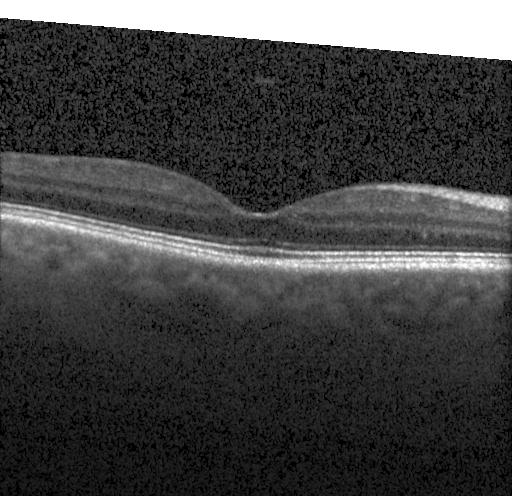
Optical coherence tomography scan. Finding: no evidence of choroidal neovascularization, diabetic macular edema, or drusen.